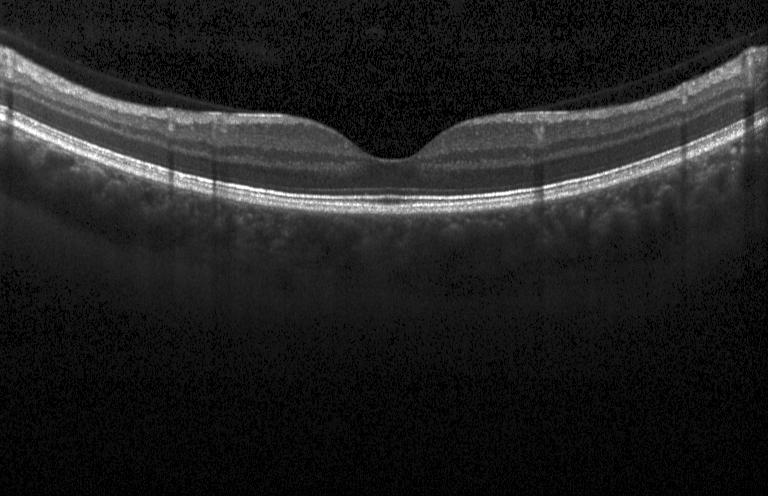
Heidelberg Spectralis OCT system, OCT B-scan, SD-OCT — Diagnosis: neither choroidal neovascularization, diabetic macular edema, nor drusen.